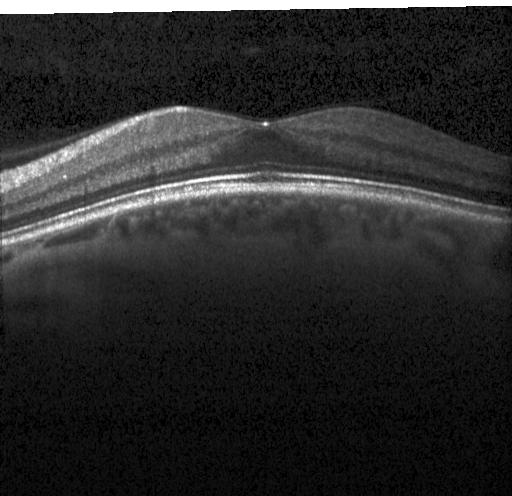
Impression: no evidence of choroidal neovascularization, diabetic macular edema, or drusen.